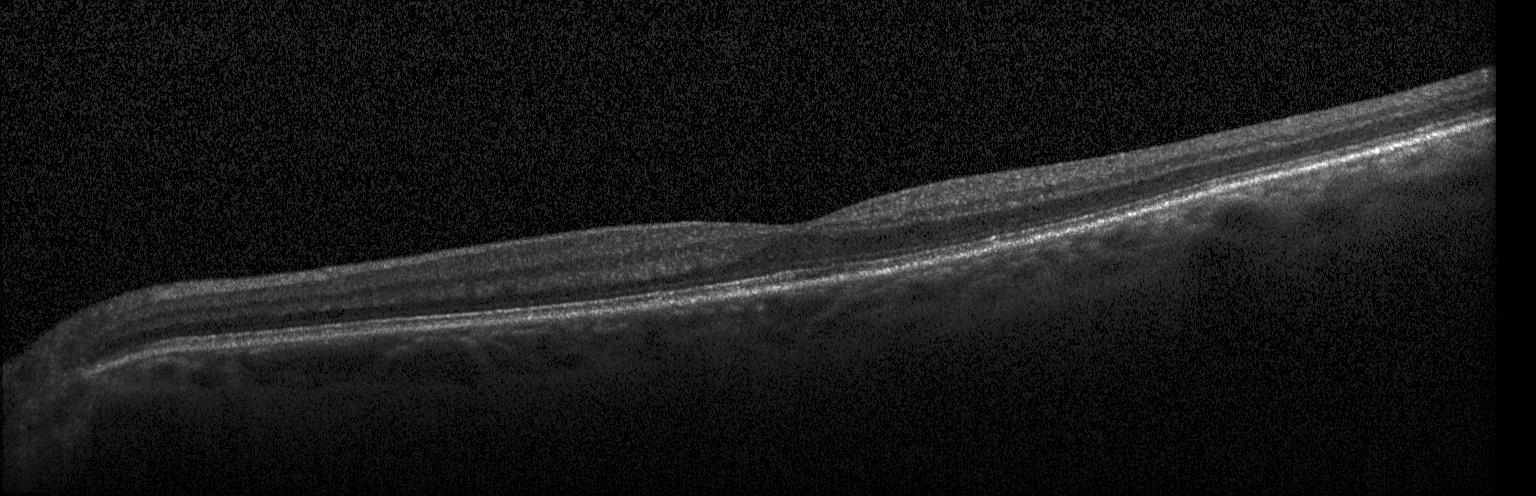 Macular OCT: no CNV, DME, or drusen.